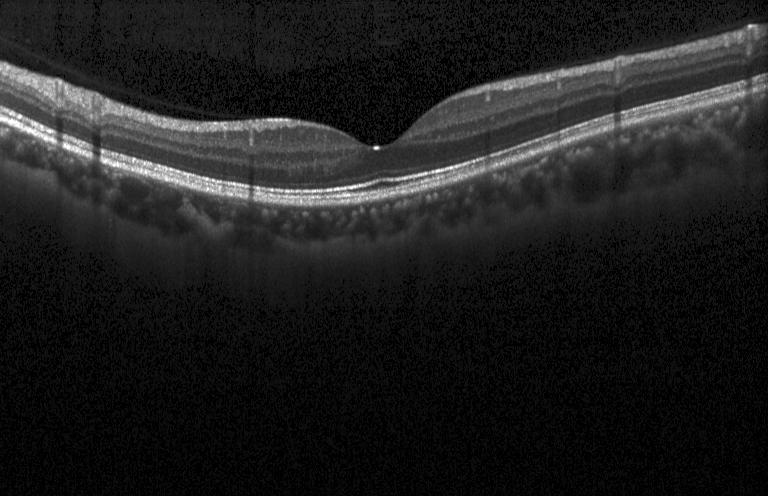

Retinal OCT B-scan.
OCT finding: no evidence of choroidal neovascularization, diabetic macular edema, or drusen.